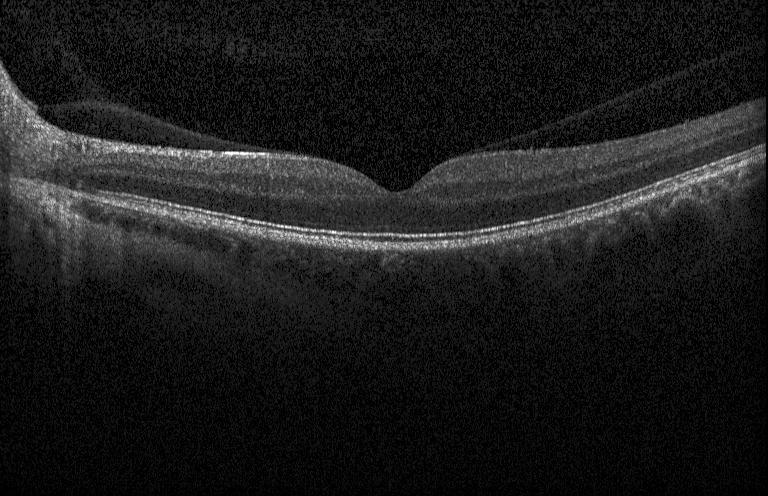
Impression: neither choroidal neovascularization, diabetic macular edema, nor drusen.